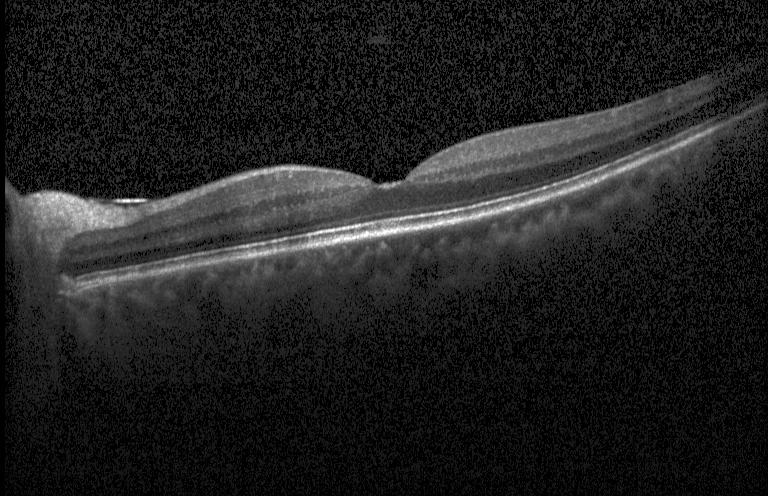 Heidelberg Spectralis OCT system. Centered on the fovea. Optical coherence tomography B-scan.
OCT finding: no CNV, no DME, and no drusen.